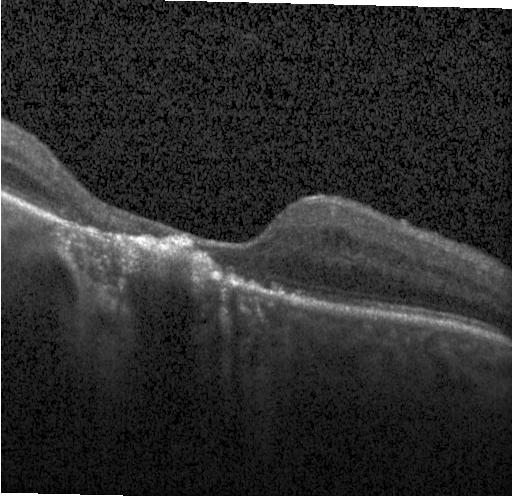
OCT finding: a choroidal neovascular membrane.